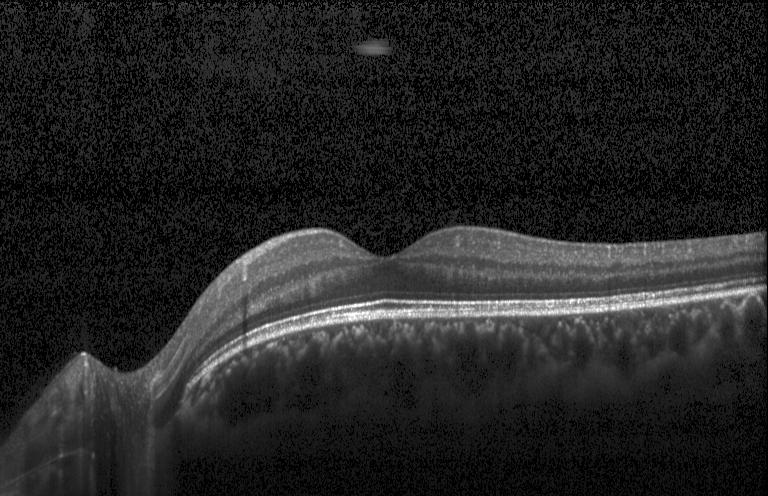

Spectral-domain OCT; macular scan; OCT B-scan.
Neither choroidal neovascularization, diabetic macular edema, nor drusen.